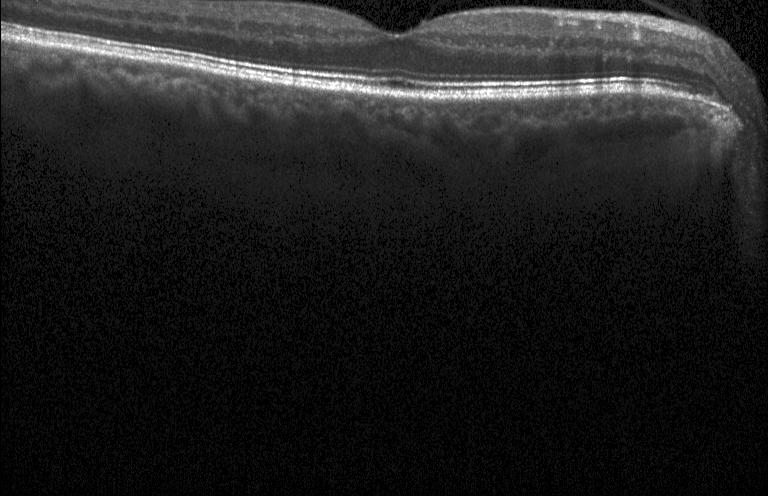
Fovea-centered · acquired on a Heidelberg Spectralis · spectral-domain optical coherence tomography · OCT line scan
Assessment: no CNV, DME, or drusen.